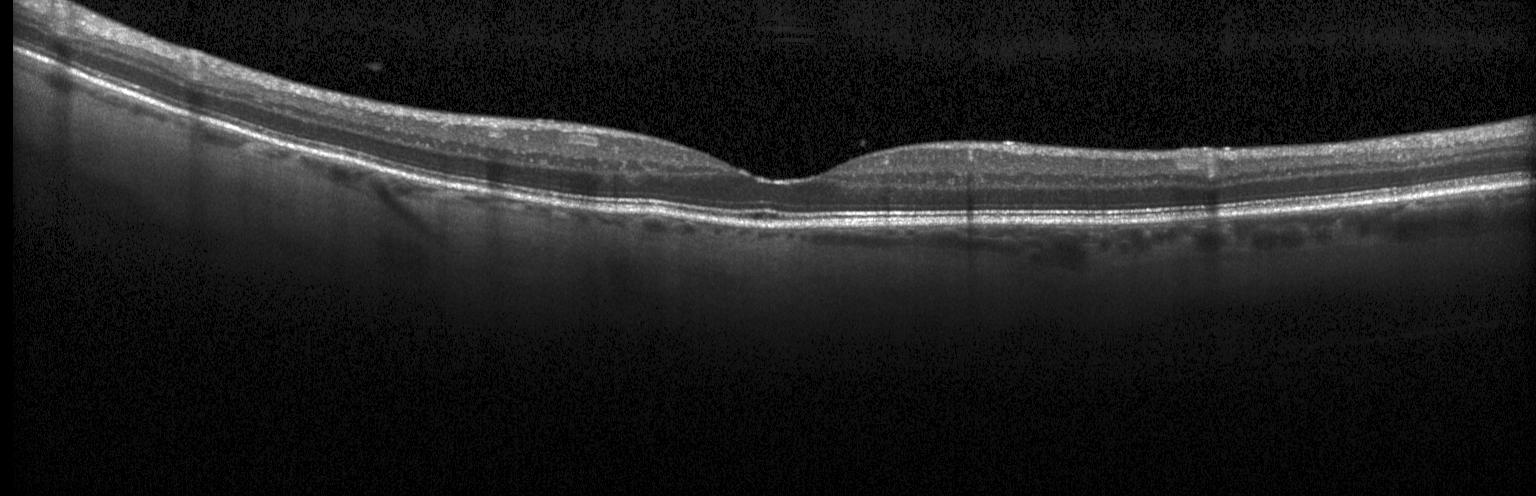

Retinal OCT B-scan — OCT finding: no evidence of choroidal neovascularization, diabetic macular edema, or drusen.